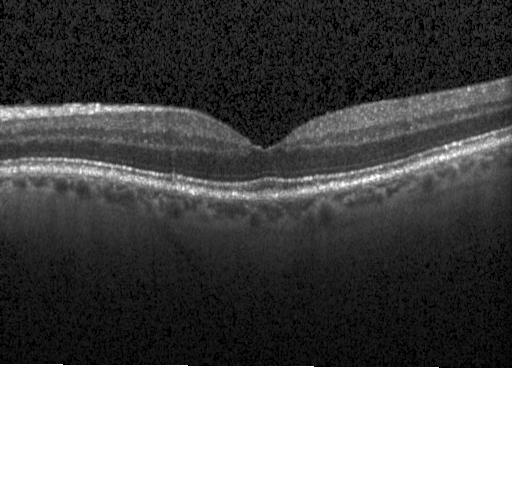
Retinal OCT cross-section. Finding: no evidence of CNV, DME, or drusen.